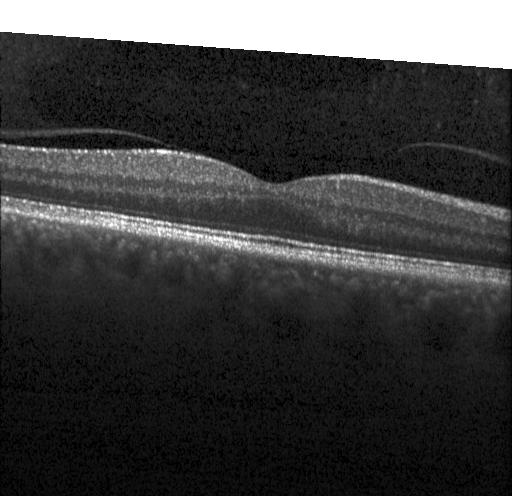 Optical coherence tomography scan — Finding: no choroidal neovascularization, no diabetic macular edema, and no drusen.